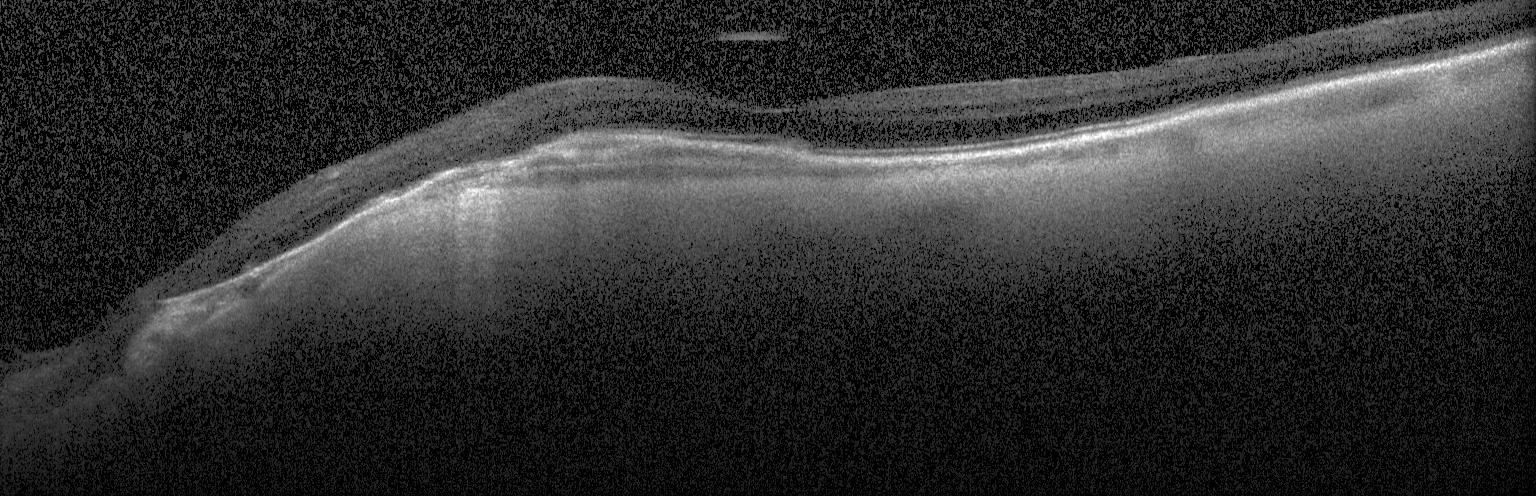
Retinal OCT cross-section. Fovea-centered
OCT finding: choroidal neovascularization.